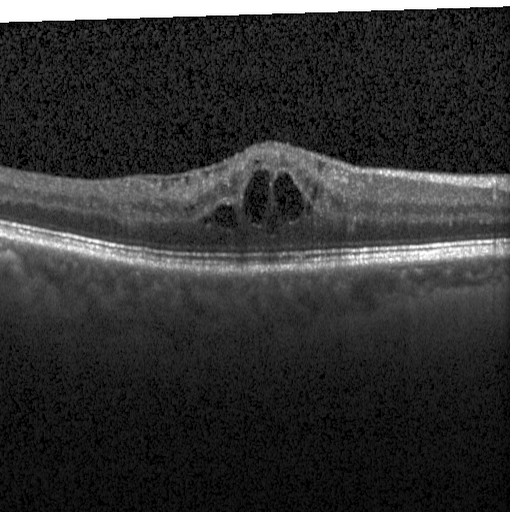
Spectral-domain optical coherence tomography · optical coherence tomography scan · horizontal scan through the fovea. Macular OCT: diabetic macular edema.